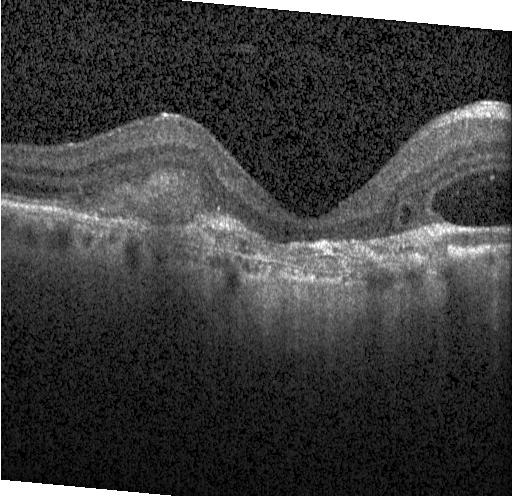
Spectral-domain OCT. Retinal OCT cross-section. Centered on the fovea. Impression: a choroidal neovascular membrane.